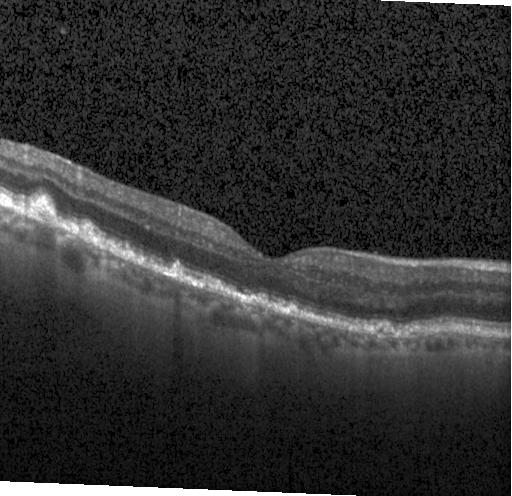 Optical coherence tomography scan, centered on the fovea, spectral-domain OCT, Heidelberg Spectralis OCT system
The scan shows multiple drusen.